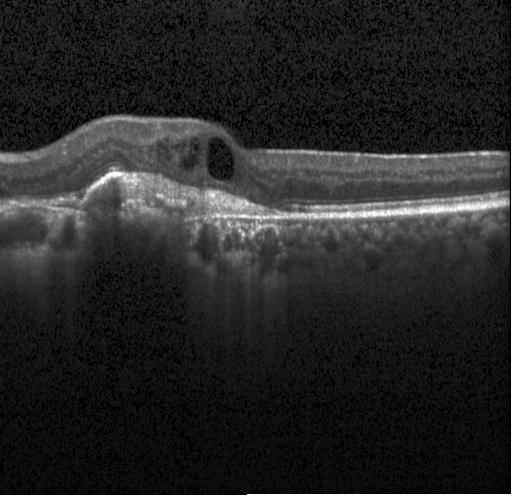

Diagnosis: choroidal neovascularization.